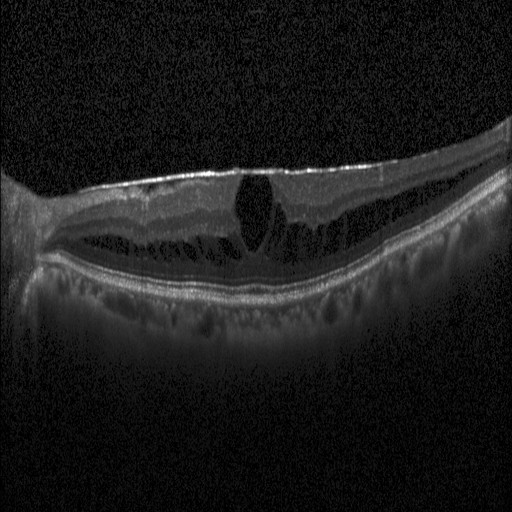
Retinal OCT B-scan; horizontal scan through the fovea; Heidelberg Spectralis OCT system
DME.